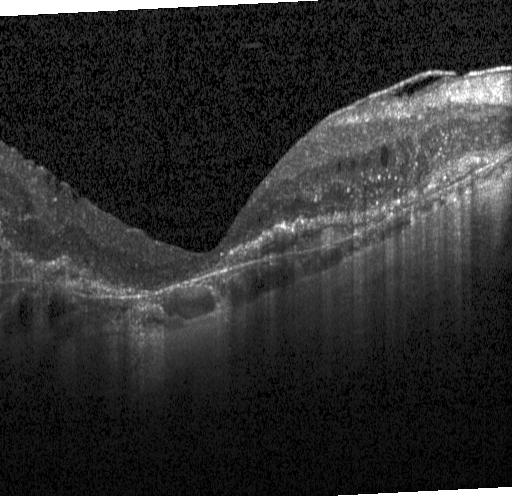
Finding: a choroidal neovascular membrane.